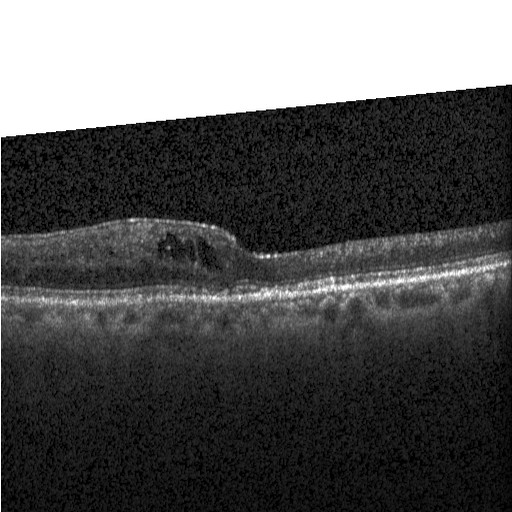
Retinal OCT B-scan. Diagnosis: diabetic macular edema.